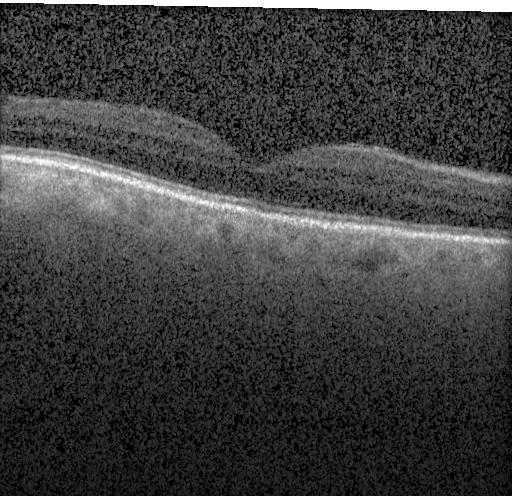 OCT B-scan showing no choroidal neovascularization, no diabetic macular edema, and no drusen.